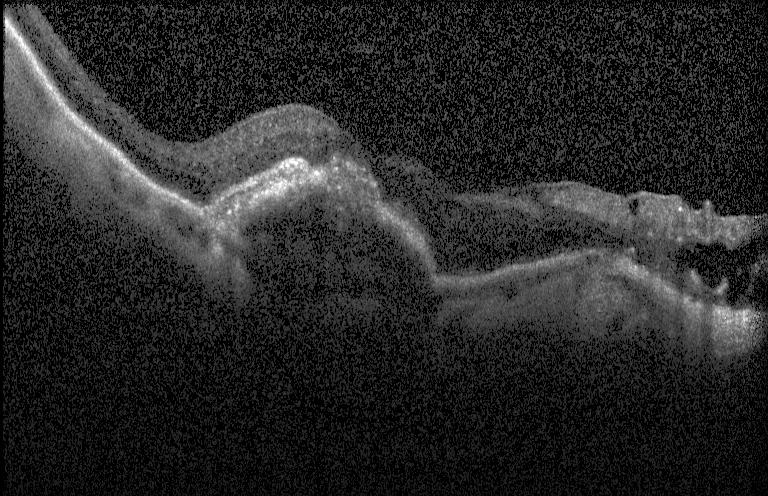 Macular OCT demonstrating a choroidal neovascular membrane.